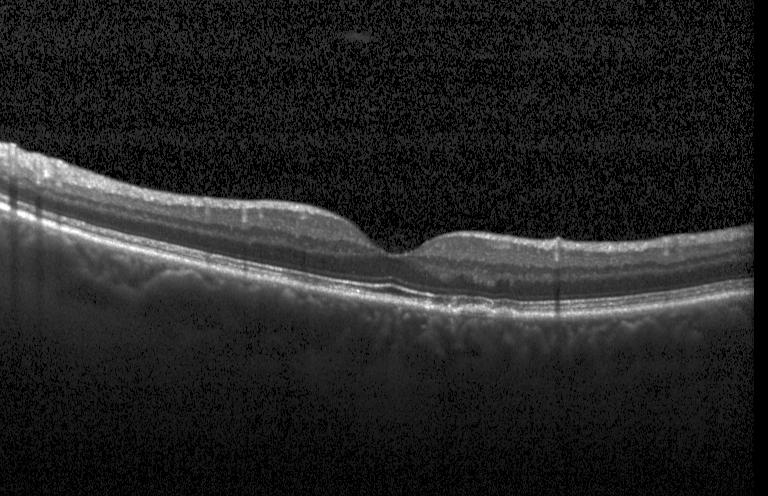
Optical coherence tomography scan.
Impression: drusen.